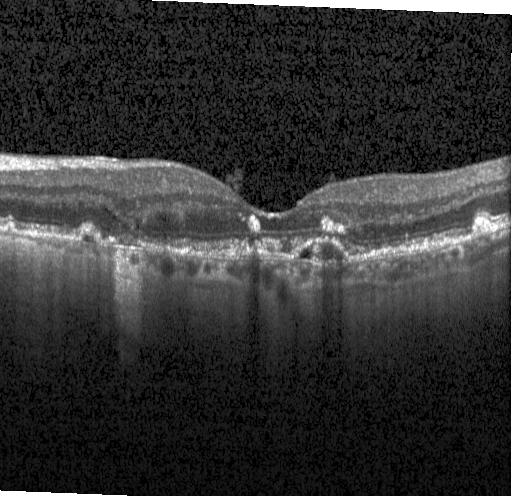
Retinal OCT B-scan — Finding: a choroidal neovascular membrane.